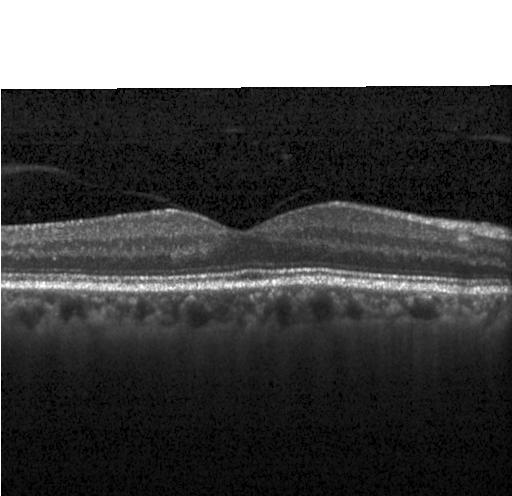
Impression: no choroidal neovascularization, no diabetic macular edema, and no drusen.